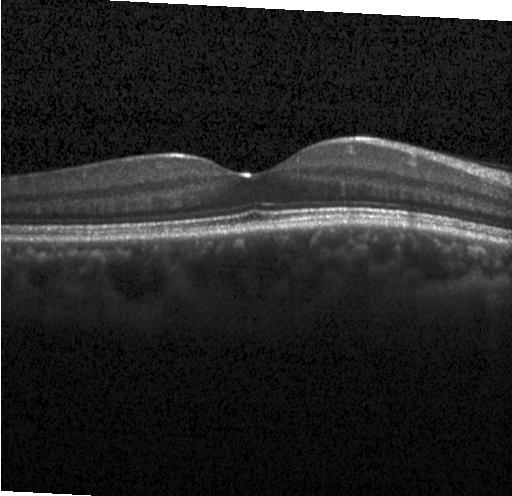

Retinal OCT cross-section — Diagnosis: no evidence of choroidal neovascularization, diabetic macular edema, or drusen.